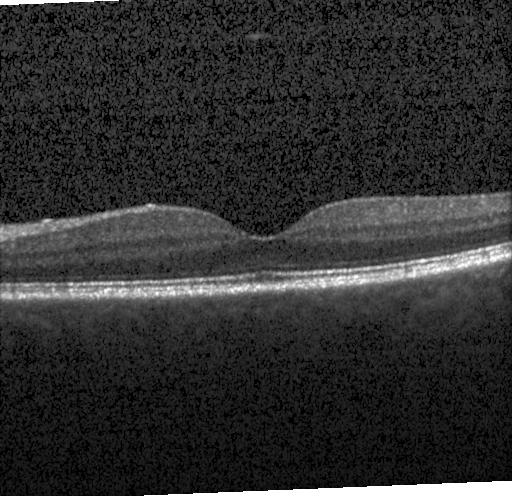 Optical coherence tomography scan. Assessment: no evidence of choroidal neovascularization, diabetic macular edema, or drusen.